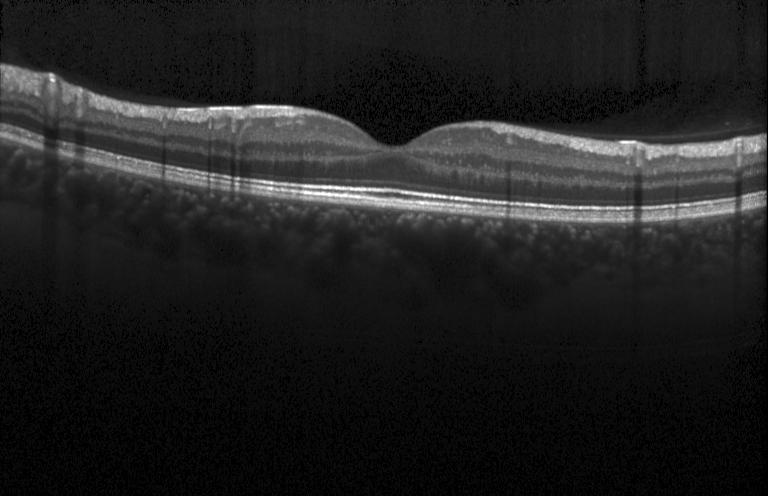

Macular OCT demonstrating neither CNV, DME, nor drusen.